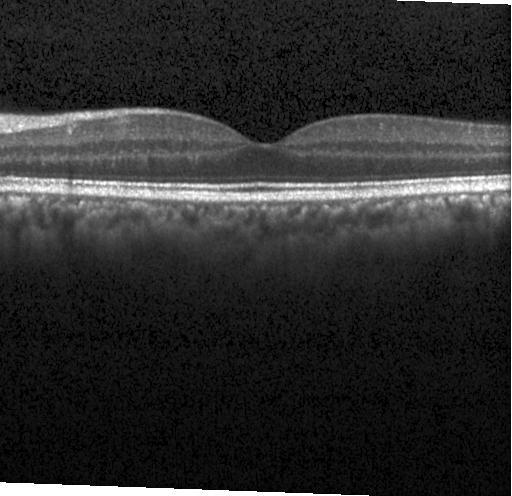 Heidelberg Spectralis OCT system, through the macula, SD-OCT, retinal OCT cross-section.
Neither choroidal neovascularization, diabetic macular edema, nor drusen.